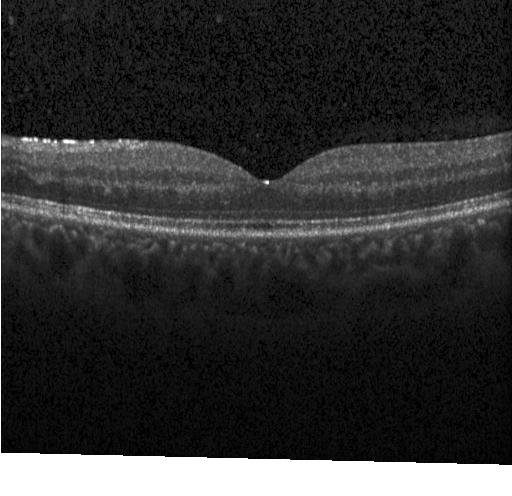 Retinal OCT cross-section — This B-scan demonstrates no choroidal neovascularization, no diabetic macular edema, and no drusen.